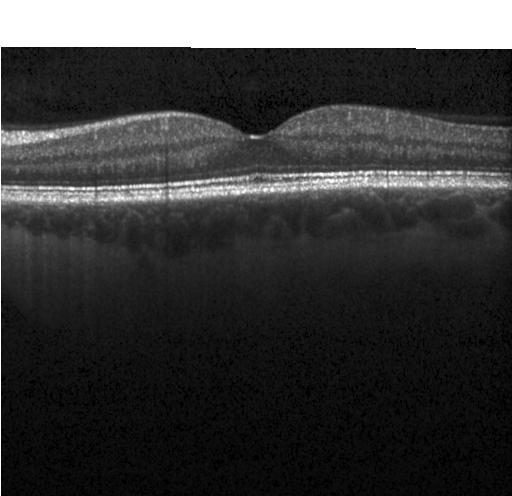 Spectral-domain OCT. Optical coherence tomography scan. Centered on the fovea. Heidelberg Spectralis OCT system
Impression: neither CNV, DME, nor drusen.